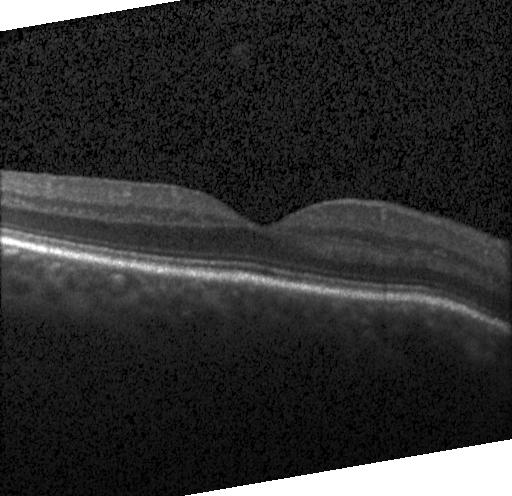

Optical coherence tomography B-scan; through the macula; acquired on a Heidelberg Spectralis; spectral-domain optical coherence tomography. The scan shows no evidence of choroidal neovascularization, diabetic macular edema, or drusen.